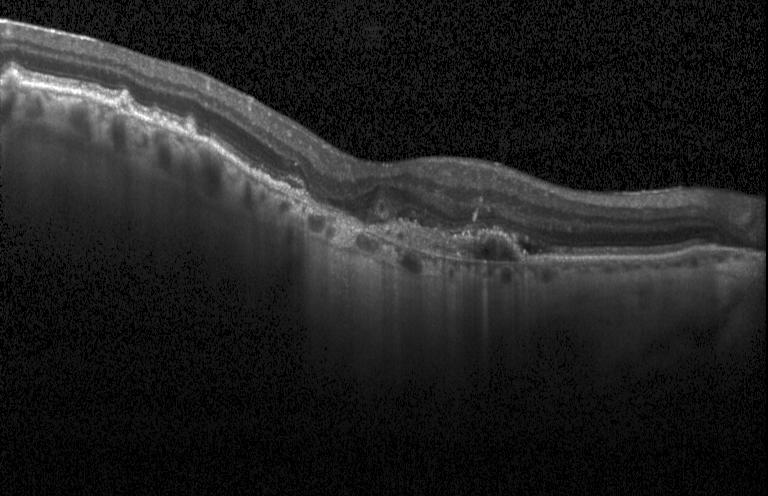

OCT B-scan; macular scan; spectral-domain OCT.
This B-scan demonstrates a choroidal neovascular membrane.